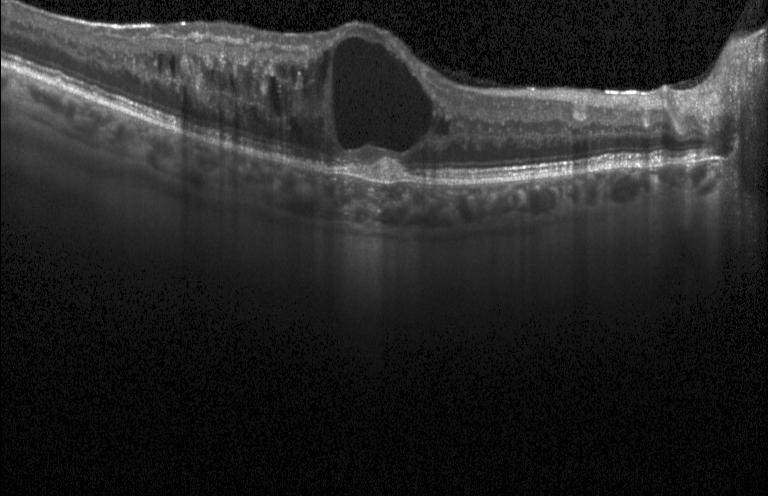
Spectral-domain OCT, through the macula, retinal OCT cross-section — Diagnosis: choroidal neovascularization (CNV).